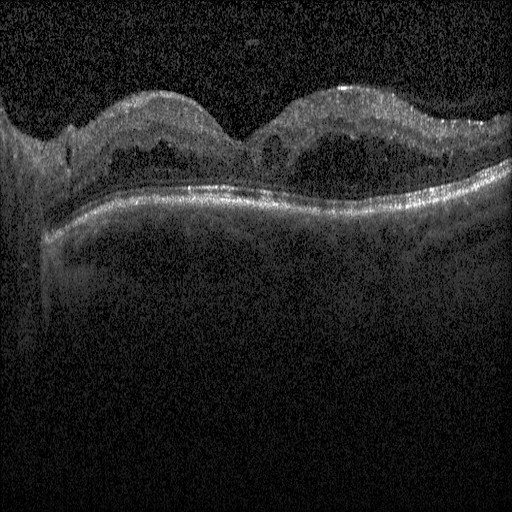
Retinal OCT cross-section
Dx: diabetic macular edema.